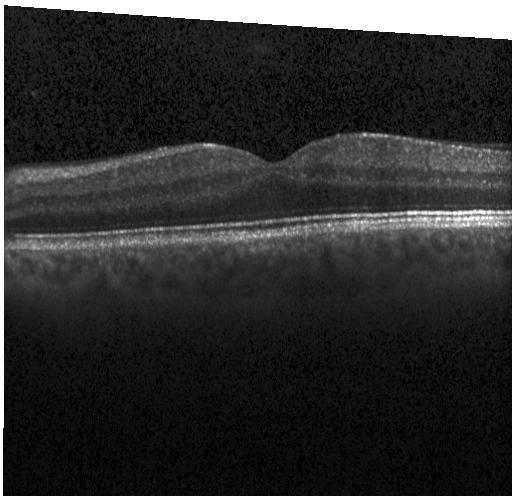
Horizontal scan through the fovea. OCT line scan. OCT finding: no evidence of CNV, DME, or drusen.